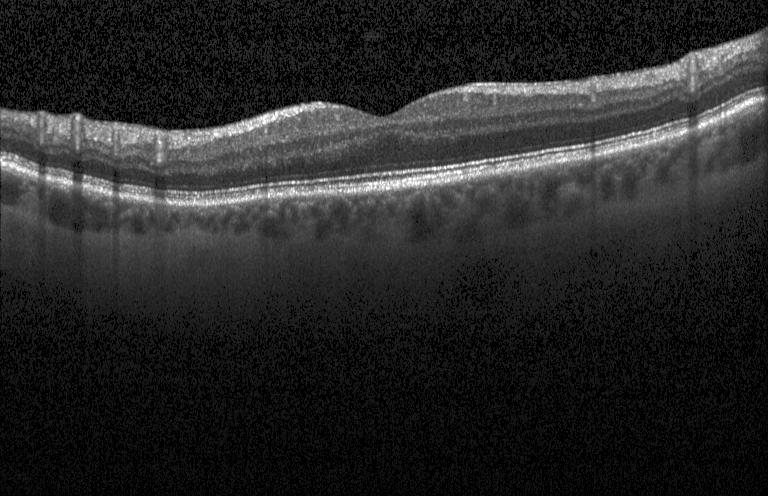
Heidelberg Spectralis OCT system; SD-OCT; optical coherence tomography B-scan; horizontal scan through the fovea. Assessment: no choroidal neovascularization, diabetic macular edema, or drusen.